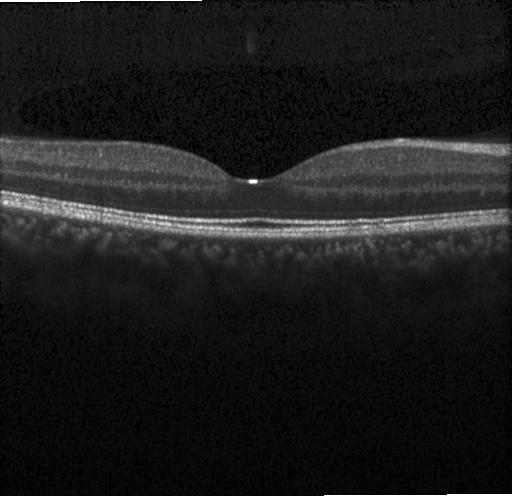 Heidelberg Spectralis. Retinal OCT cross-section. Fovea-centered. Spectral-domain OCT
The scan shows no CNV, no DME, and no drusen.